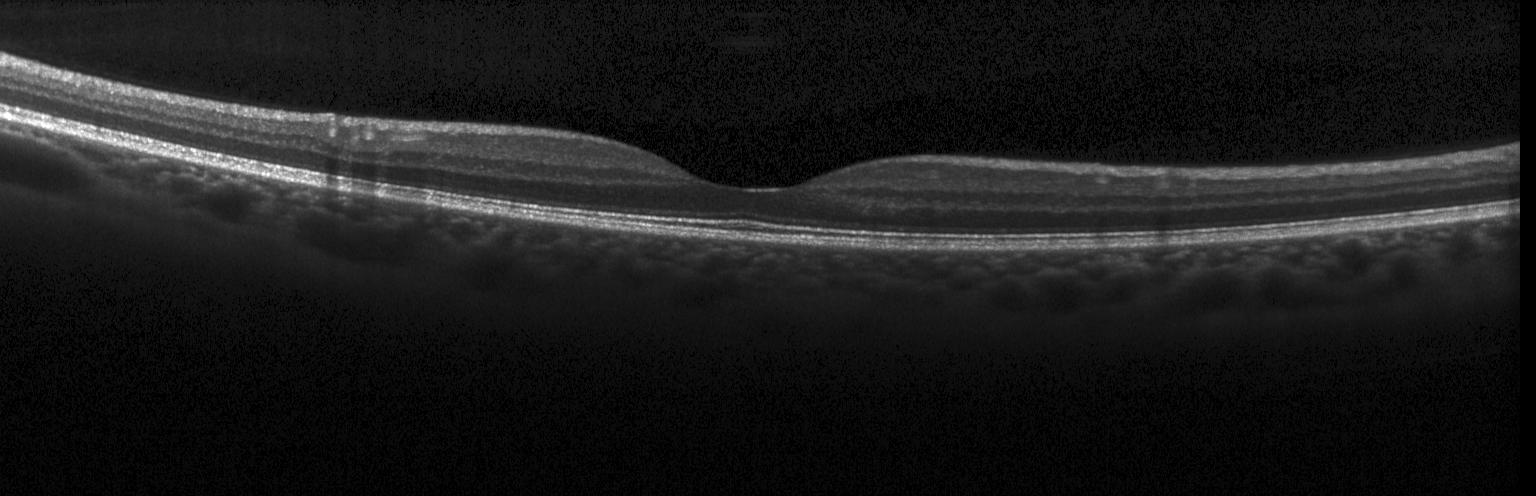

Dx: no choroidal neovascularization, no diabetic macular edema, and no drusen.